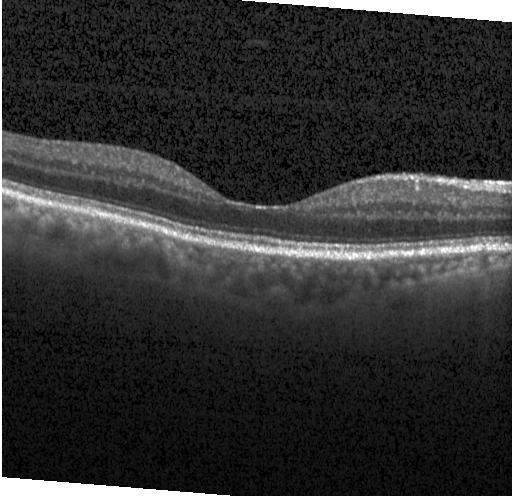 Retinal OCT cross-section. Finding: no choroidal neovascularization, diabetic macular edema, or drusen.